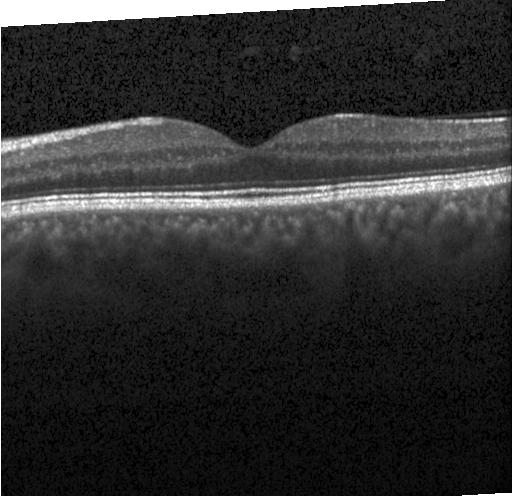 Acquired on a Heidelberg Spectralis · spectral-domain OCT · optical coherence tomography scan · centered on the fovea.
Diagnosis: neither choroidal neovascularization, diabetic macular edema, nor drusen.